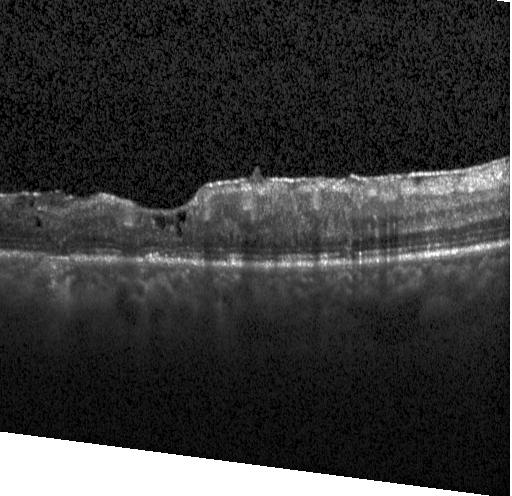
Macular scan, optical coherence tomography scan, Heidelberg Spectralis, spectral-domain OCT
Impression: DME.